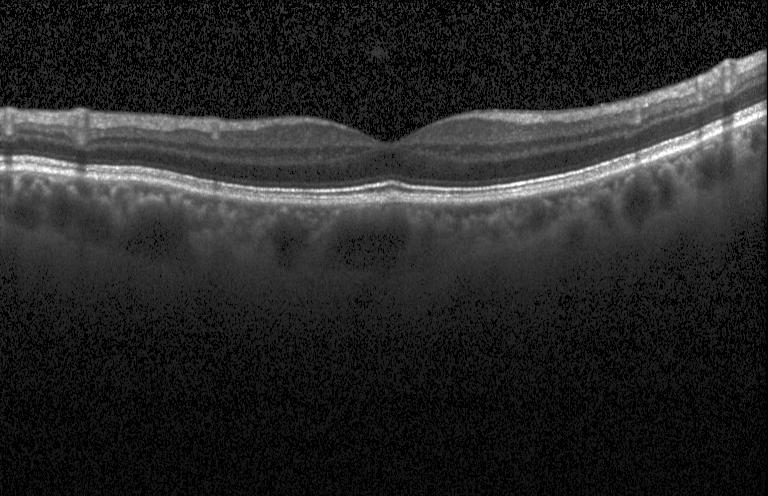 Retinal OCT cross-section; centered on the fovea.
Assessment: neither choroidal neovascularization, diabetic macular edema, nor drusen.